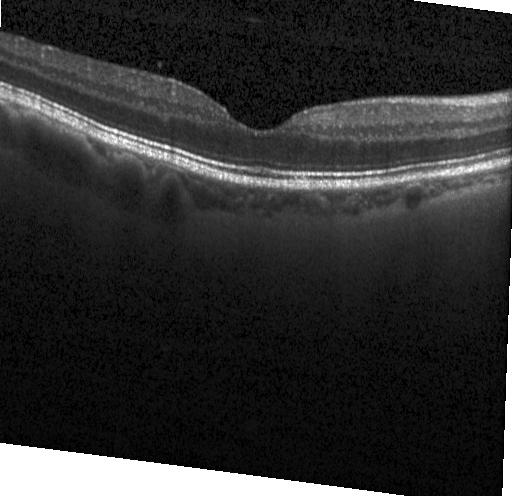
Neither choroidal neovascularization, diabetic macular edema, nor drusen.